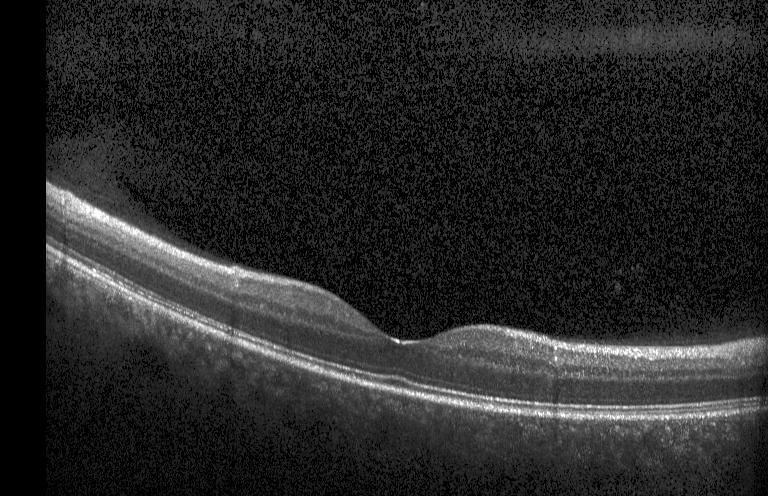

Spectral-domain optical coherence tomography · horizontal scan through the fovea · instrument: Heidelberg Spectralis · optical coherence tomography scan — Macular OCT: neither choroidal neovascularization, diabetic macular edema, nor drusen.